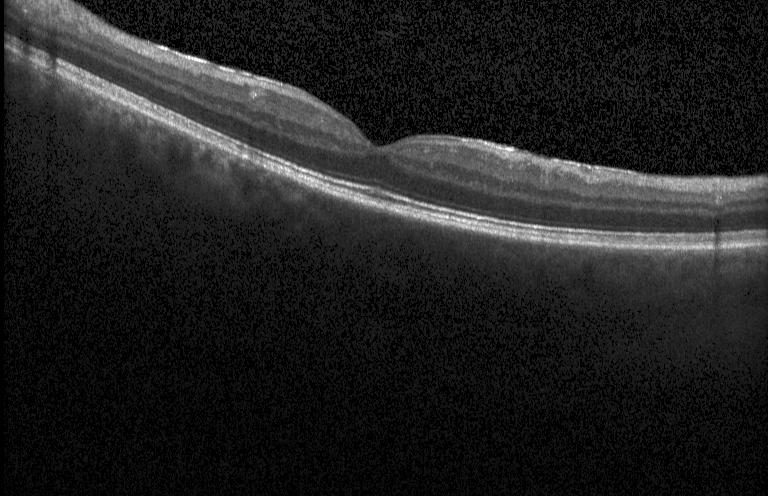
Acquired on a Heidelberg Spectralis · macular scan · SD-OCT · OCT B-scan — Impression: no choroidal neovascularization, no diabetic macular edema, and no drusen.